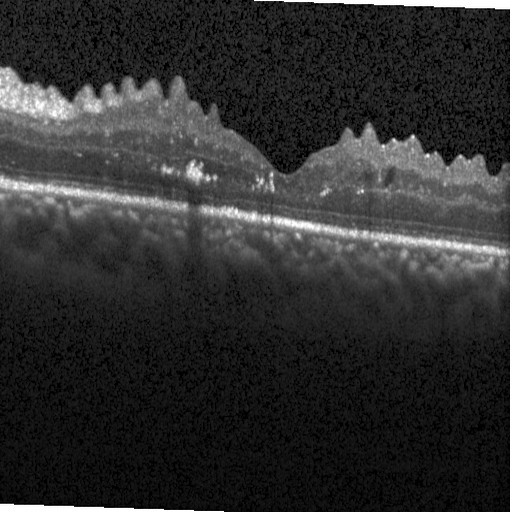 Retinal OCT cross-section. Instrument: Heidelberg Spectralis
Dx: DME.